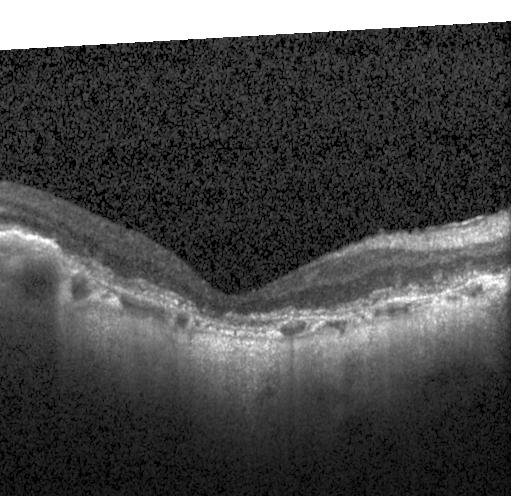

OCT line scan. SD-OCT
Diagnosis: a choroidal neovascular membrane.